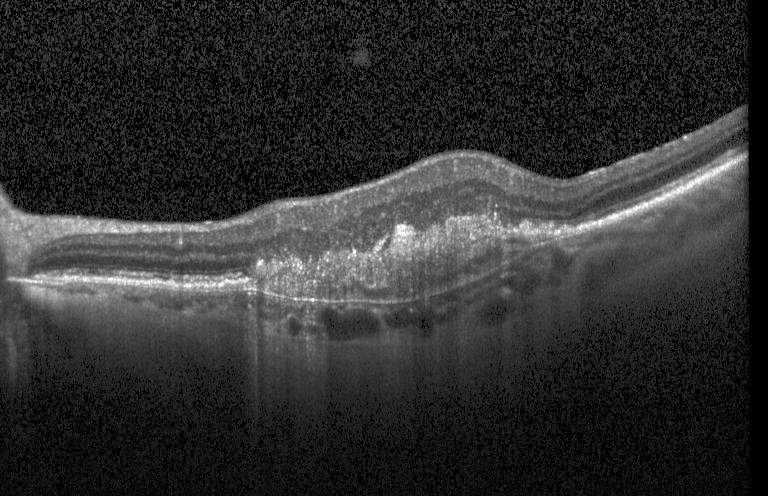

Macular OCT demonstrating choroidal neovascularization.